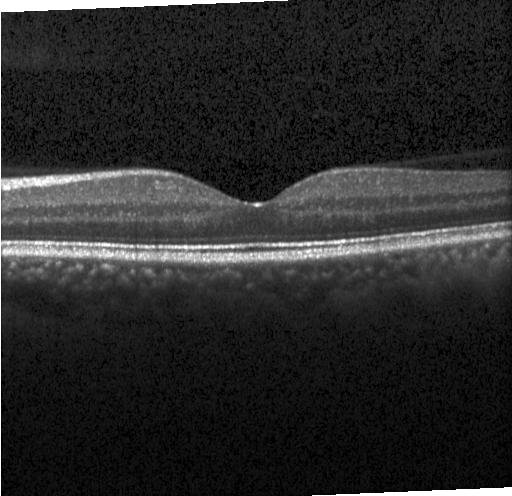
OCT scan showing no CNV, DME, or drusen.